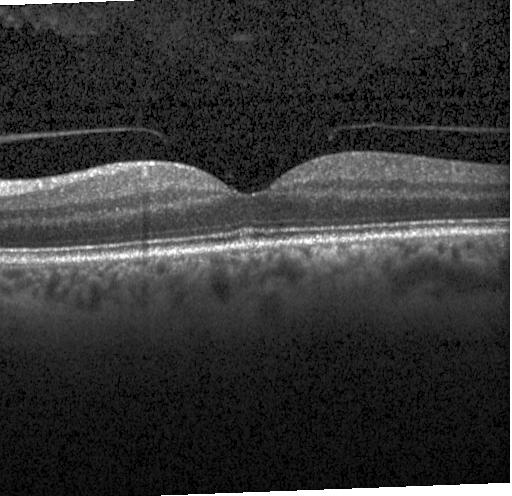 Horizontal scan through the fovea, OCT B-scan.
The scan shows neither choroidal neovascularization, diabetic macular edema, nor drusen.